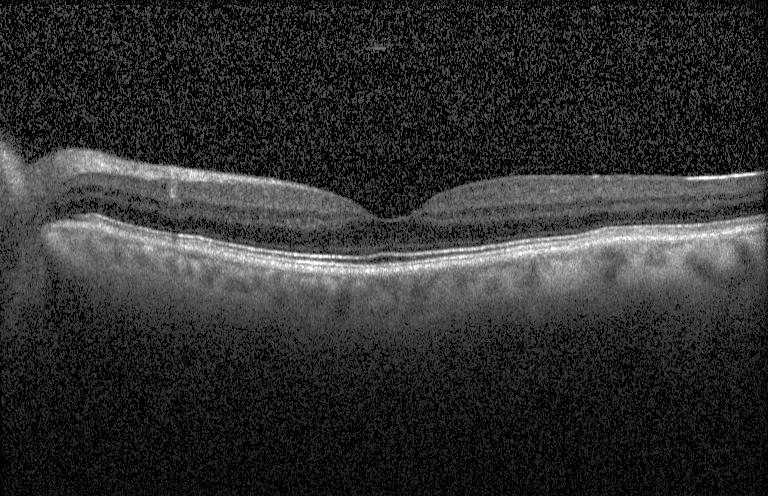

Dx: no choroidal neovascularization, no diabetic macular edema, and no drusen.